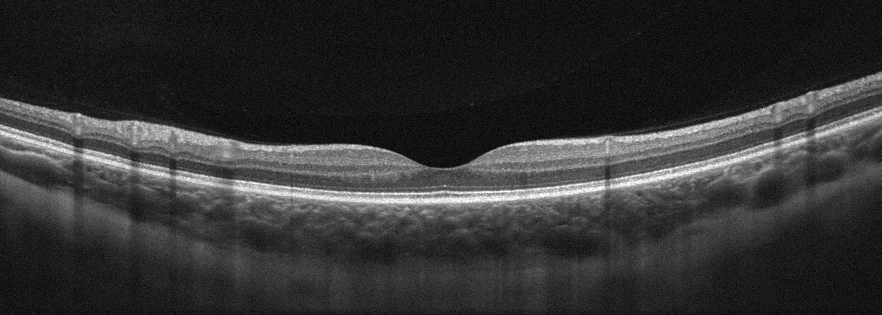 Through the macula, Optovue Avanti RTVue XR, optical coherence tomography scan.
This B-scan demonstrates absence of AMD, DME, ERM, RAO, RVO, and vitreomacular interface disease.